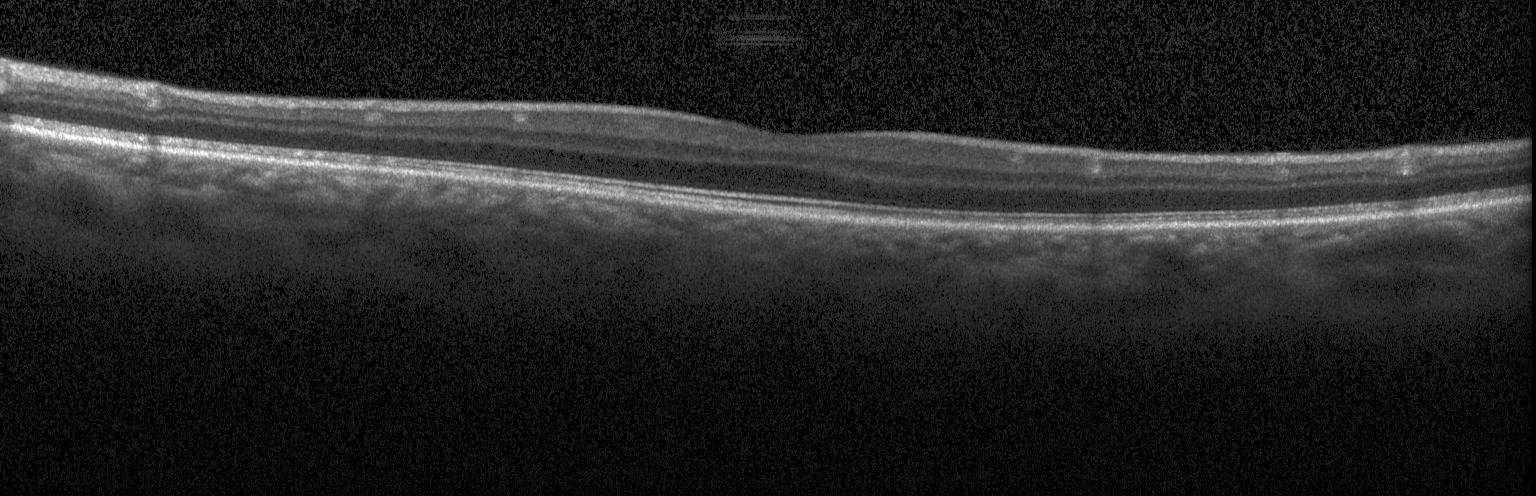

Assessment: no CNV, no DME, and no drusen.